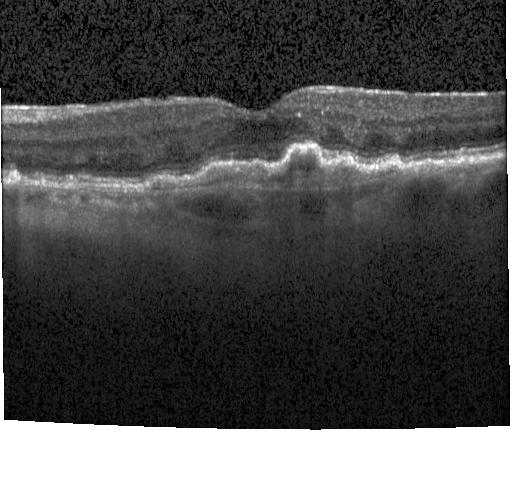
Diagnosis: a choroidal neovascular membrane.